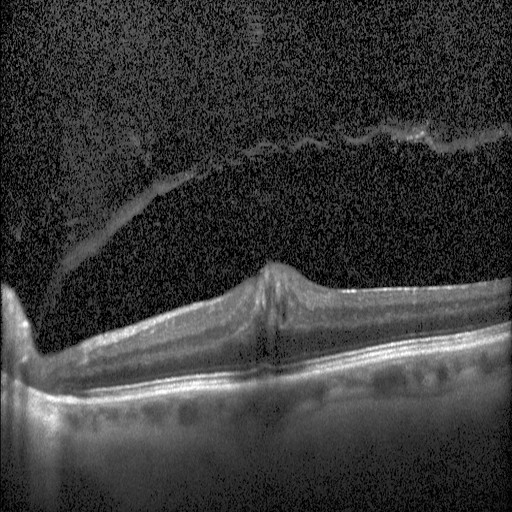

Optical coherence tomography B-scan; Heidelberg Spectralis
DME.